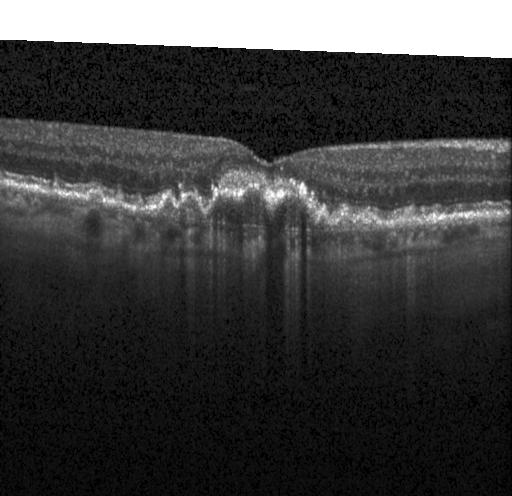
OCT finding: a choroidal neovascular membrane.